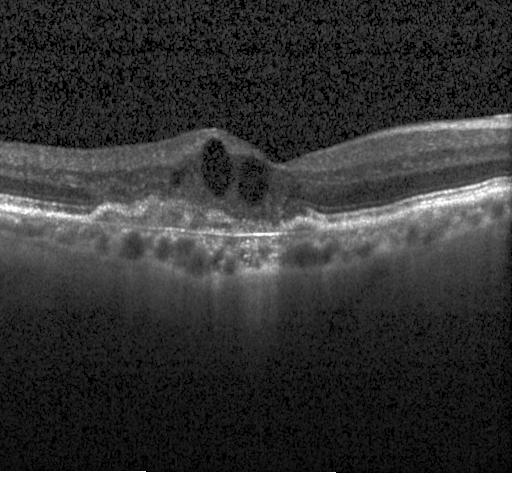 OCT B-scan; spectral-domain OCT.
Dx: choroidal neovascularization (CNV).